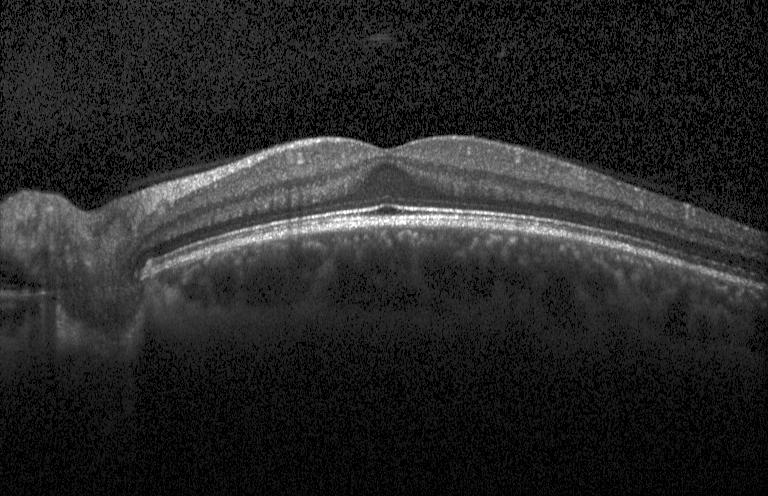
Dx: no choroidal neovascularization, diabetic macular edema, or drusen.